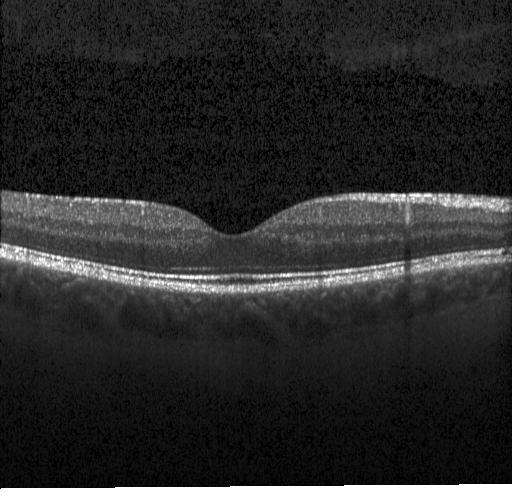 OCT scan showing no evidence of choroidal neovascularization, diabetic macular edema, or drusen.